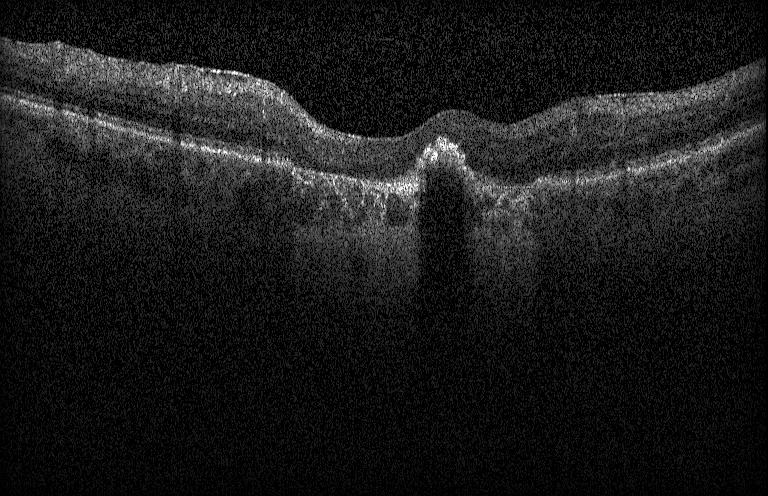
Optical coherence tomography B-scan.
A choroidal neovascular membrane.